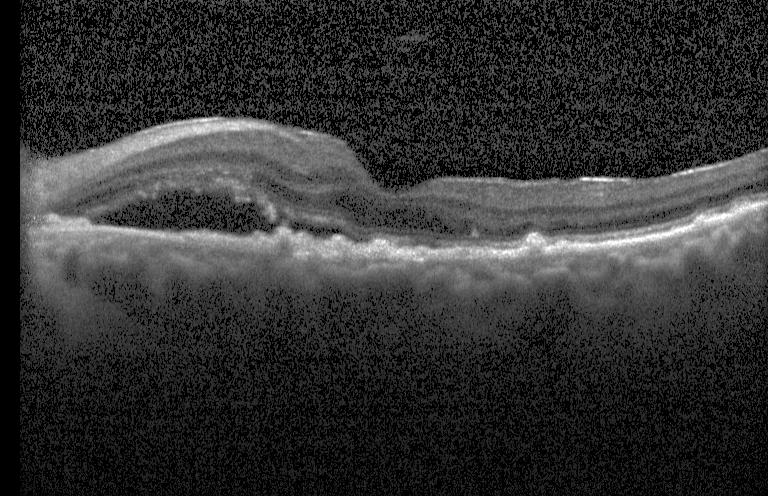 Dx: a choroidal neovascular membrane.